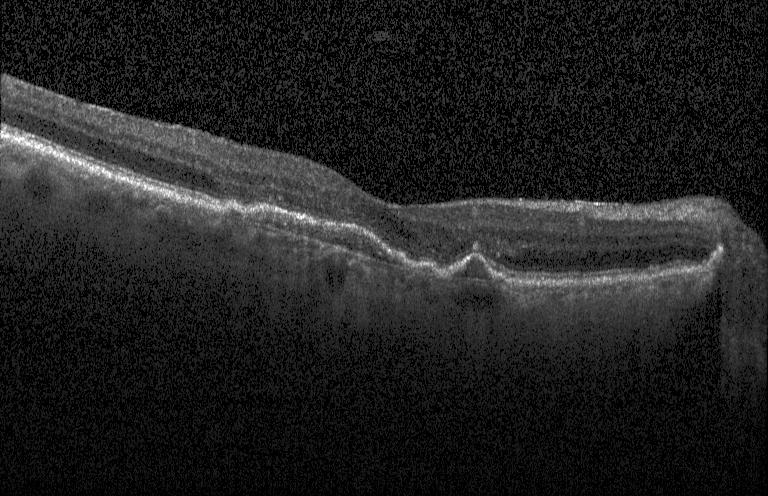 Centered on the fovea; optical coherence tomography B-scan; acquired on a Heidelberg Spectralis.
Finding: CNV.